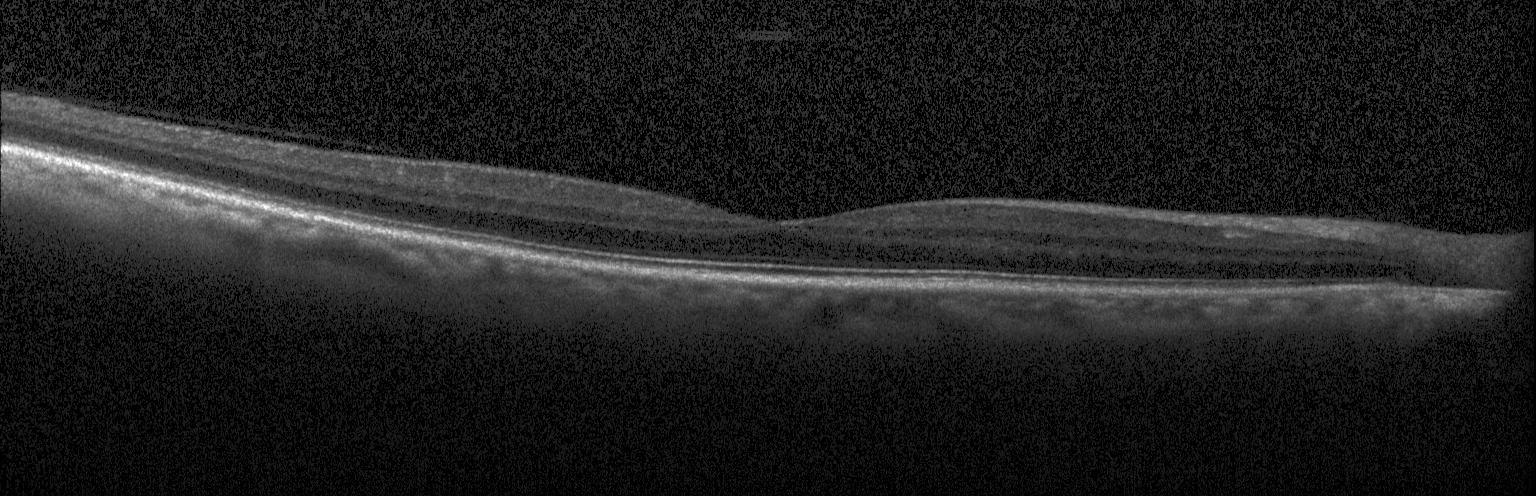

Macular OCT: neither choroidal neovascularization, diabetic macular edema, nor drusen.